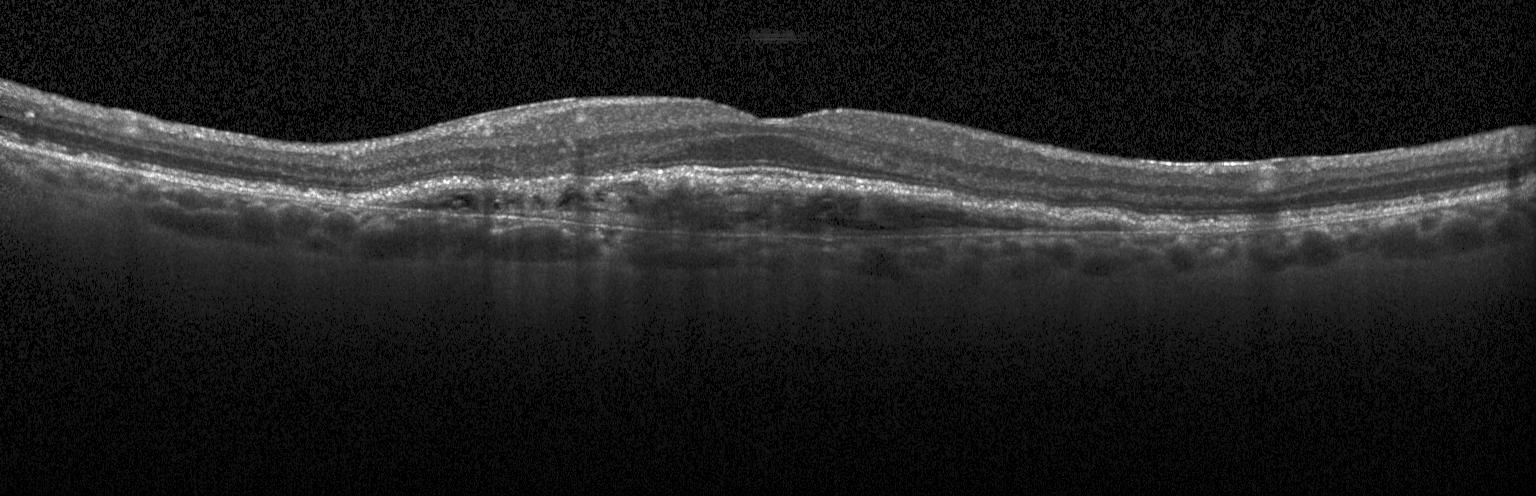

SD-OCT. OCT line scan.
Macular OCT: CNV.